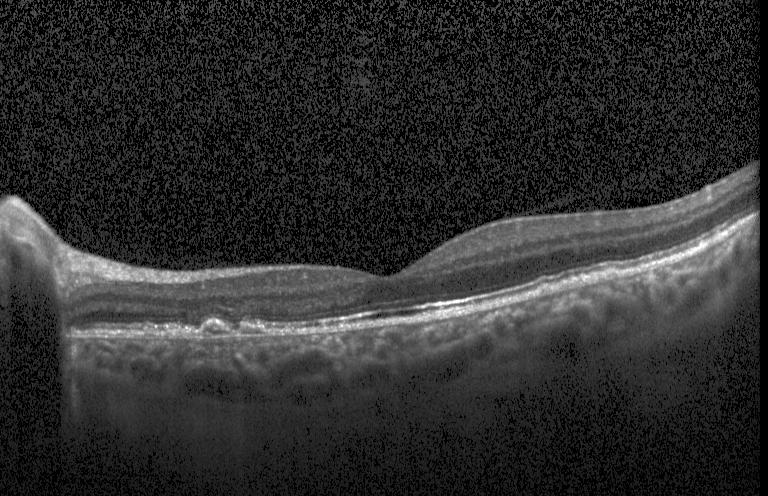
OCT B-scan, SD-OCT — Finding: choroidal neovascularization.